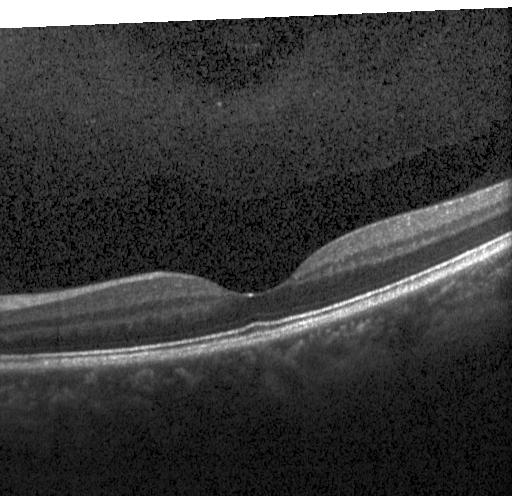
Retinal OCT cross-section, centered on the fovea, SD-OCT
This B-scan demonstrates neither CNV, DME, nor drusen.